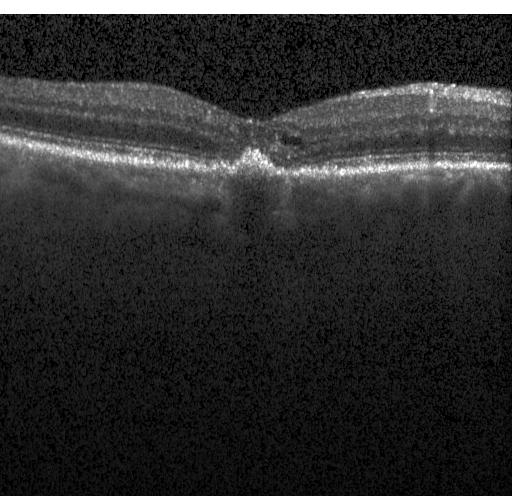
Fovea-centered · spectral-domain OCT · Heidelberg Spectralis OCT system · optical coherence tomography B-scan. This B-scan demonstrates a choroidal neovascular membrane.